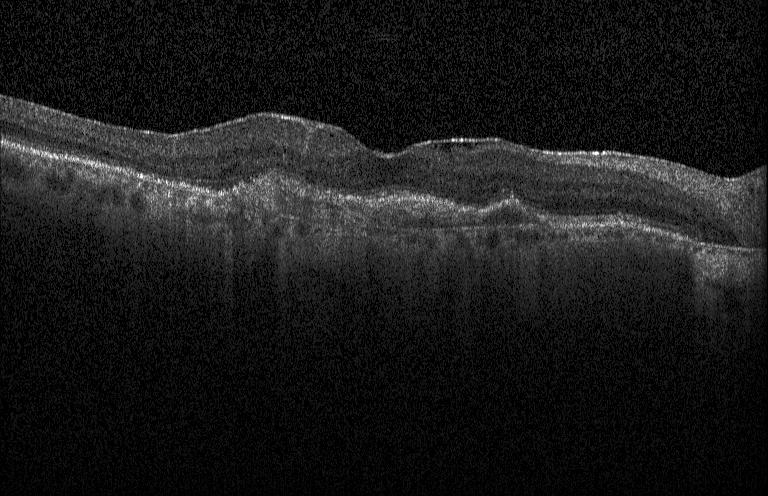 OCT B-scan showing a choroidal neovascular membrane.